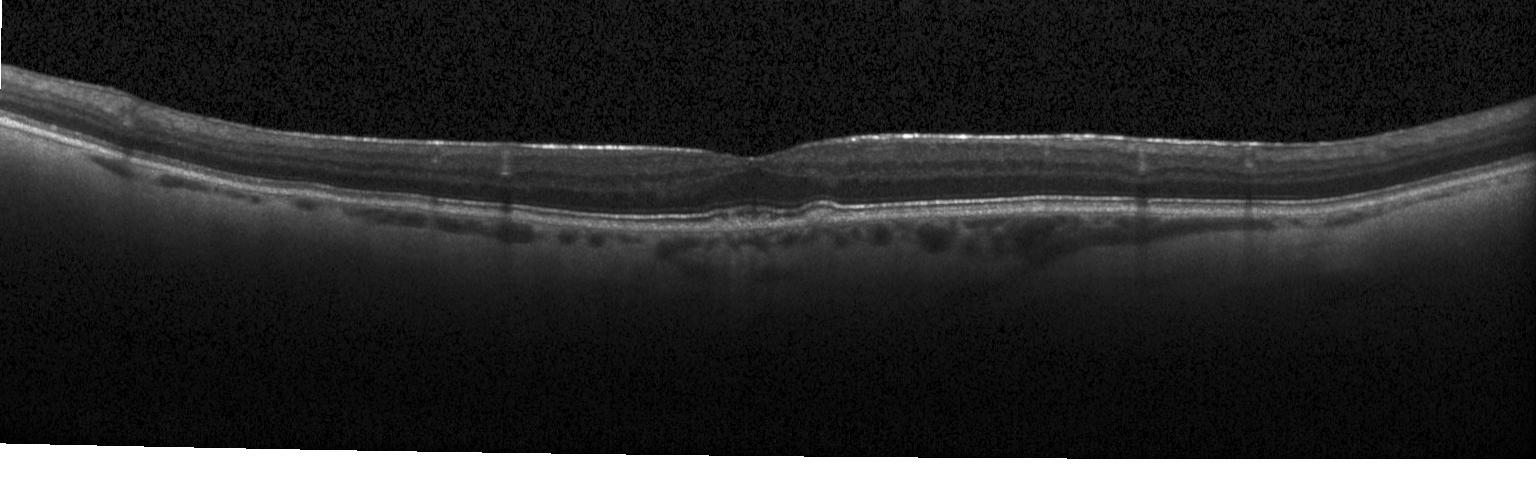 Spectral-domain optical coherence tomography, optical coherence tomography scan. Macular OCT: drusen.